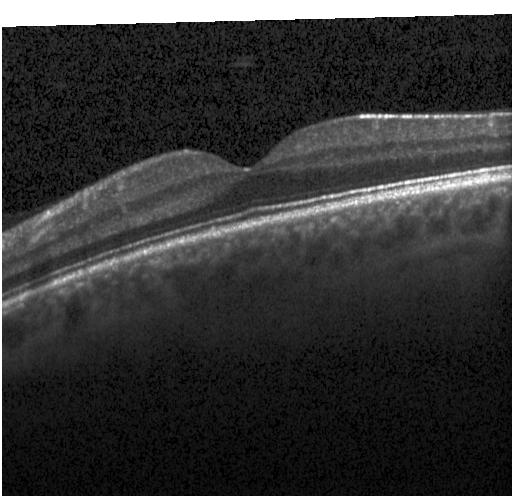
Acquired on a Heidelberg Spectralis · centered on the fovea · retinal OCT B-scan.
The scan shows no evidence of CNV, DME, or drusen.